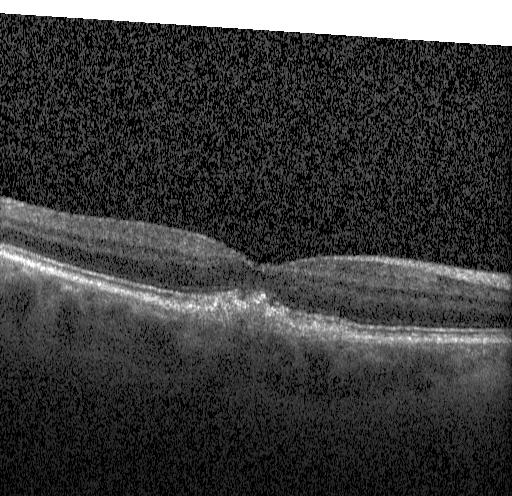 SD-OCT; horizontal scan through the fovea; Heidelberg Spectralis OCT system; retinal OCT B-scan.
Diagnosis: multiple drusen.